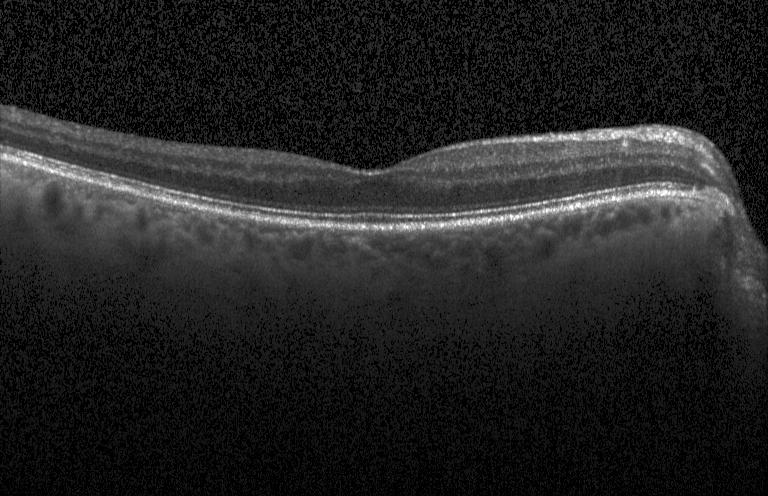
Heidelberg Spectralis; centered on the fovea; optical coherence tomography B-scan; SD-OCT — This B-scan demonstrates no choroidal neovascularization, no diabetic macular edema, and no drusen.